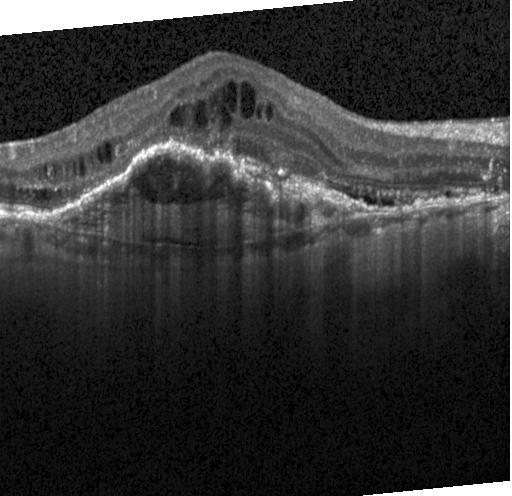

OCT scan showing choroidal neovascularization.